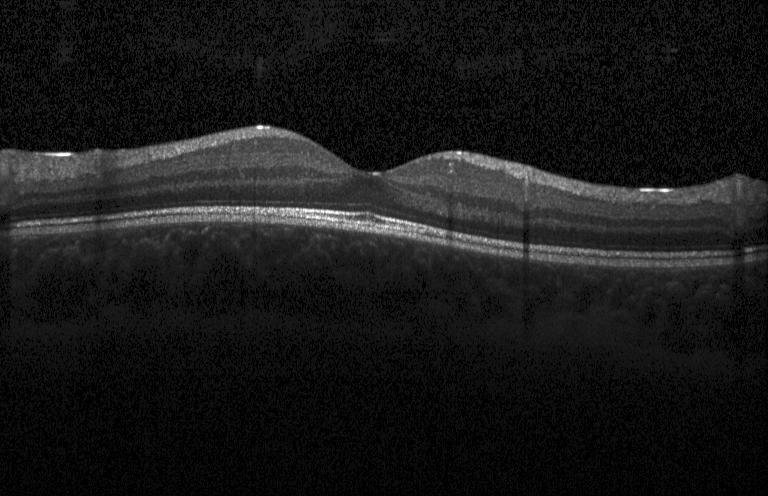 Retinal OCT B-scan. Through the macula. Instrument: Heidelberg Spectralis. Impression: no evidence of CNV, DME, or drusen.